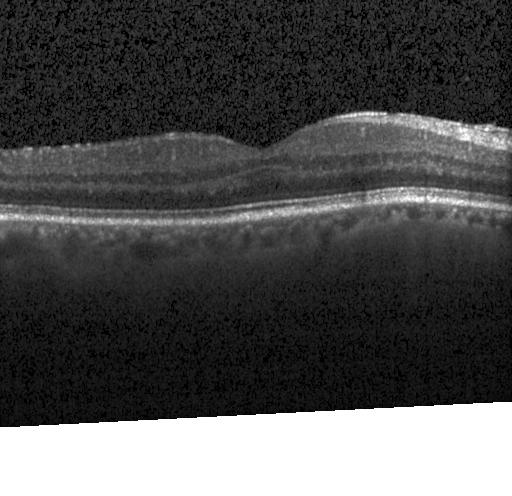

Finding: neither CNV, DME, nor drusen.